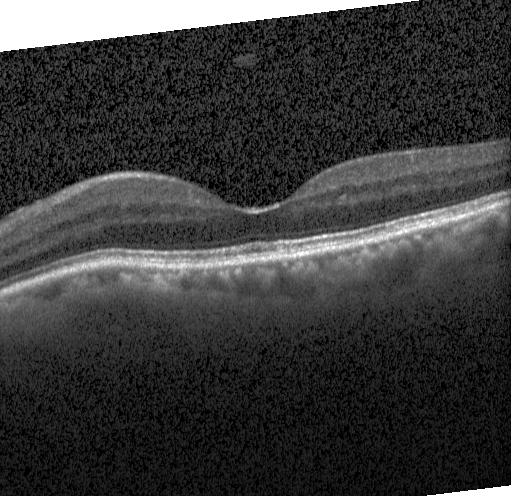 Heidelberg Spectralis OCT system, horizontal scan through the fovea, spectral-domain optical coherence tomography, OCT B-scan. Dx: neither choroidal neovascularization, diabetic macular edema, nor drusen.